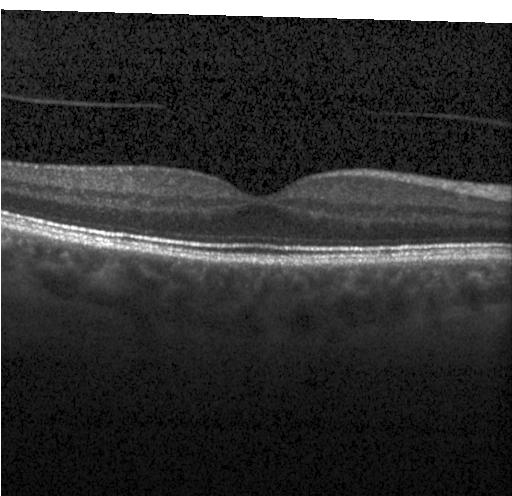

Optical coherence tomography scan; spectral-domain optical coherence tomography; Heidelberg Spectralis.
Impression: no evidence of choroidal neovascularization, diabetic macular edema, or drusen.